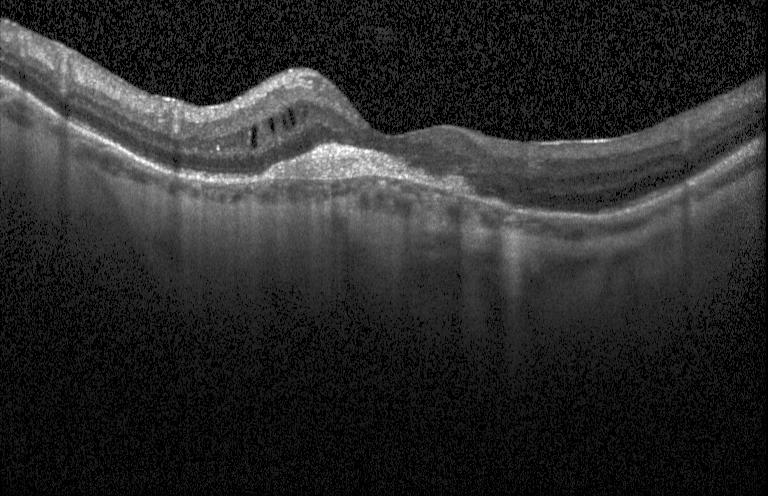 Heidelberg Spectralis; optical coherence tomography B-scan; SD-OCT. Macular OCT: choroidal neovascularization (CNV).